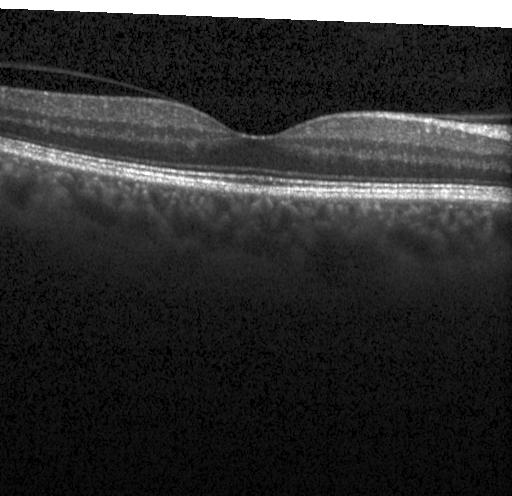 Heidelberg Spectralis OCT system, optical coherence tomography scan, SD-OCT, fovea-centered. Impression: no CNV, DME, or drusen.